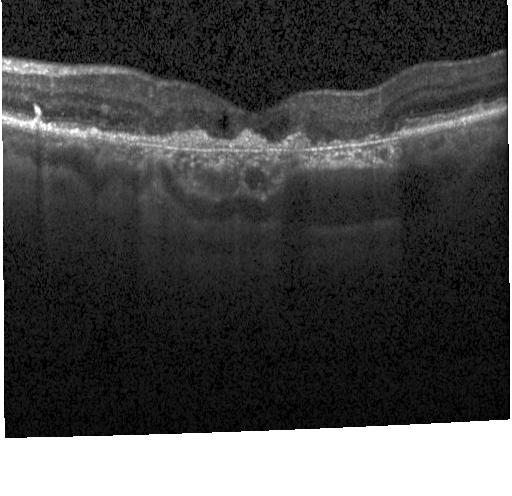
Heidelberg Spectralis OCT system; spectral-domain optical coherence tomography; macular scan; OCT line scan.
This B-scan demonstrates CNV.